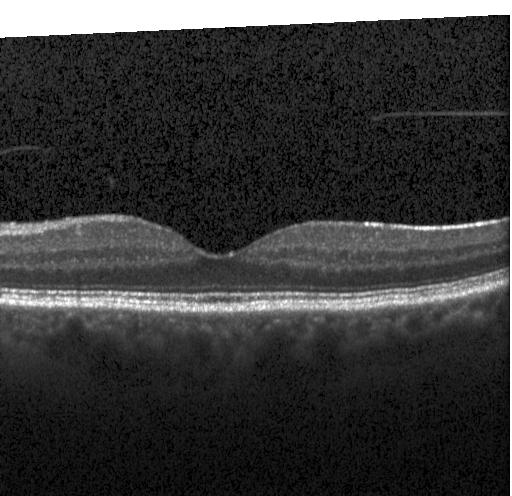
OCT finding: no CNV, no DME, and no drusen.